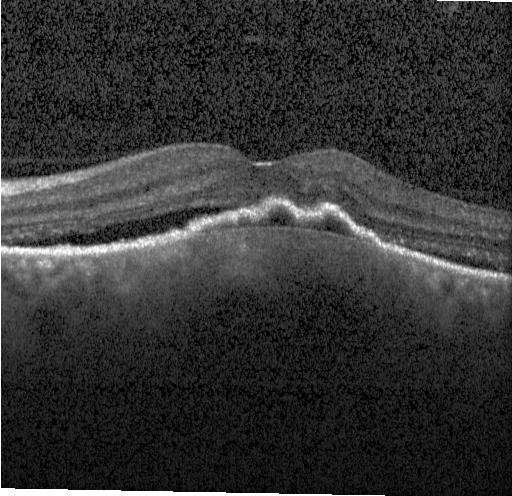
Finding: choroidal neovascularization (CNV).